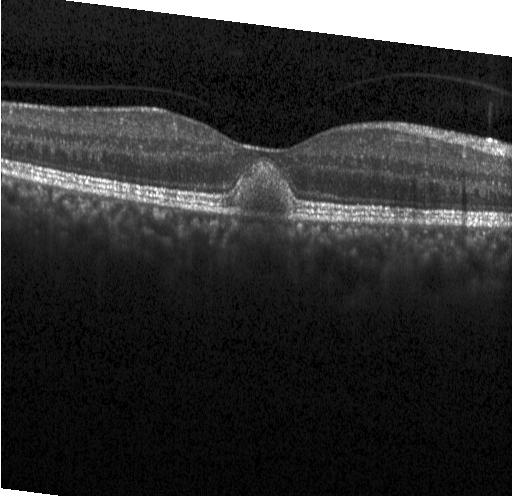

Optical coherence tomography scan. Finding: choroidal neovascularization.